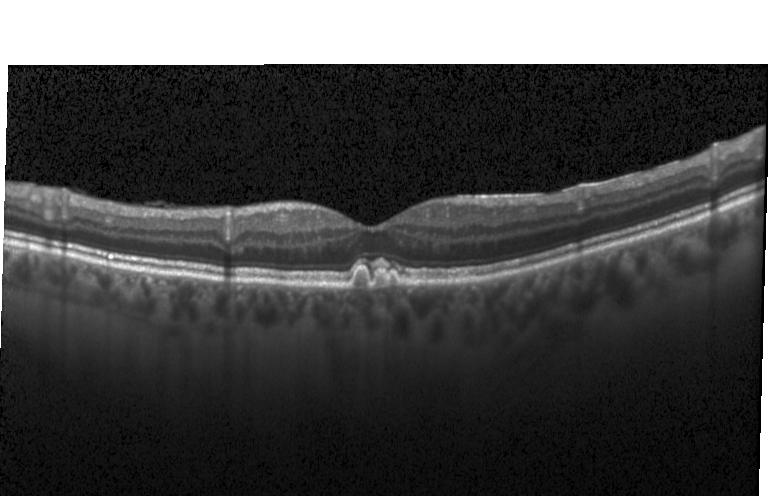
Horizontal scan through the fovea, OCT B-scan, spectral-domain OCT — This B-scan demonstrates multiple drusen.